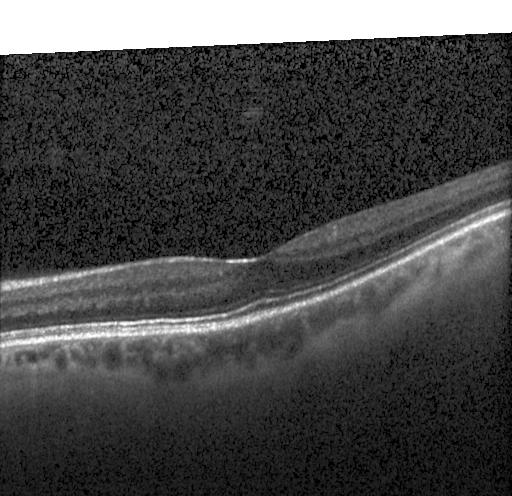

Assessment: no CNV, no DME, and no drusen.